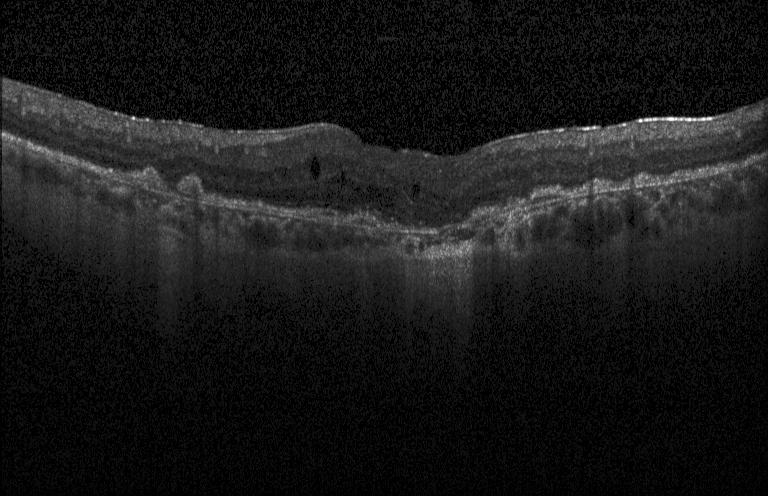

Instrument: Heidelberg Spectralis, horizontal scan through the fovea, spectral-domain optical coherence tomography, OCT line scan. Finding: a choroidal neovascular membrane.